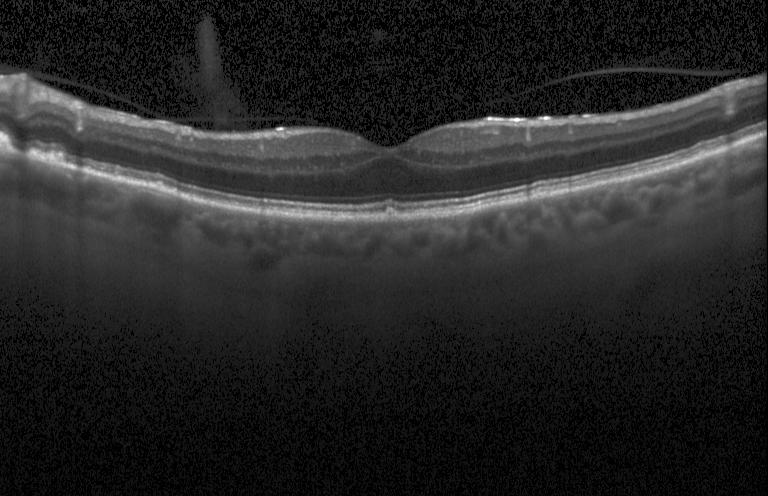 The scan shows no choroidal neovascularization, no diabetic macular edema, and no drusen.